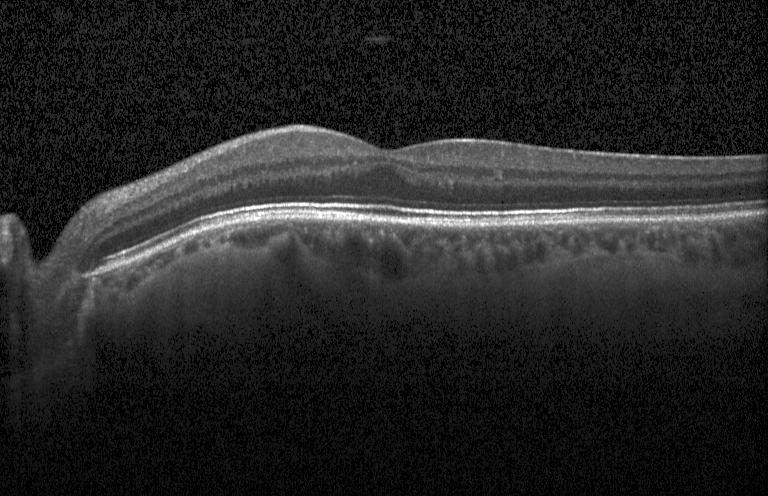 Optical coherence tomography B-scan, instrument: Heidelberg Spectralis
No evidence of choroidal neovascularization, diabetic macular edema, or drusen.